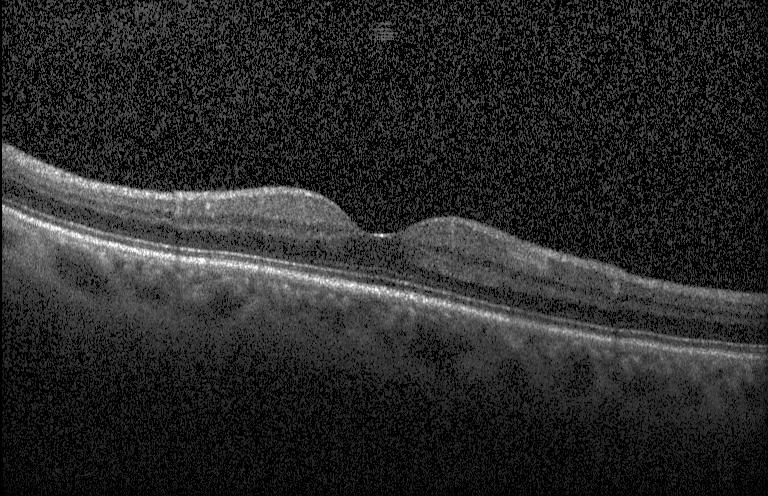 Spectral-domain OCT B-scan: no evidence of choroidal neovascularization, diabetic macular edema, or drusen.